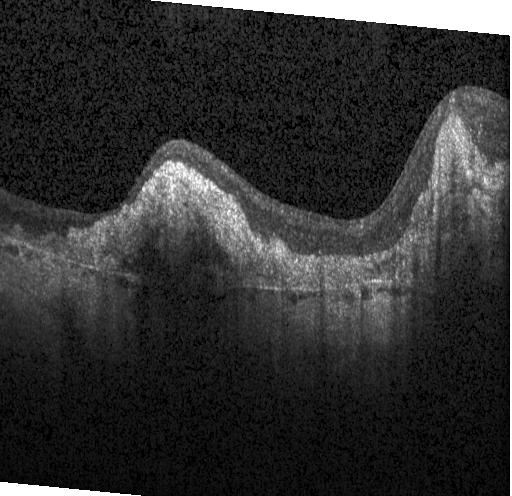 OCT scan showing choroidal neovascularization (CNV).